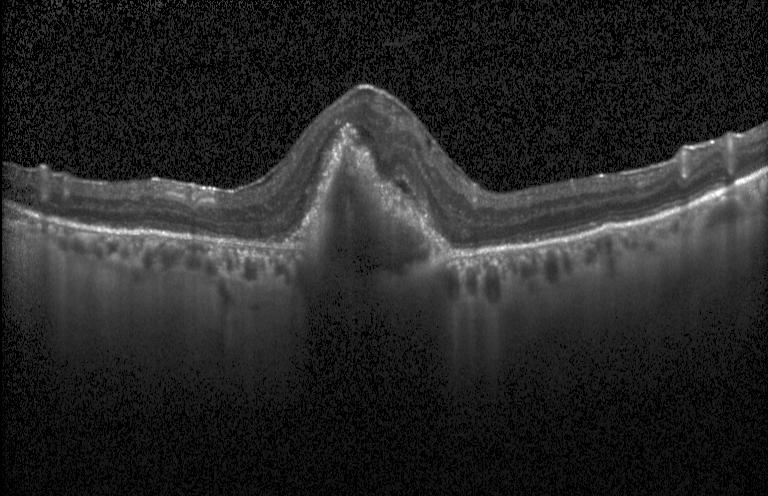
Macular OCT: CNV.